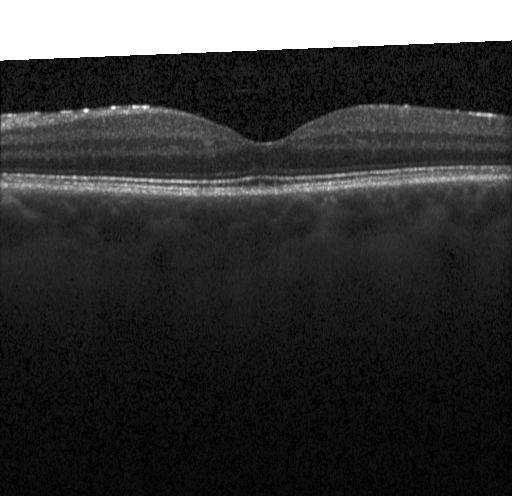 OCT line scan · fovea-centered. Impression: no choroidal neovascularization, diabetic macular edema, or drusen.